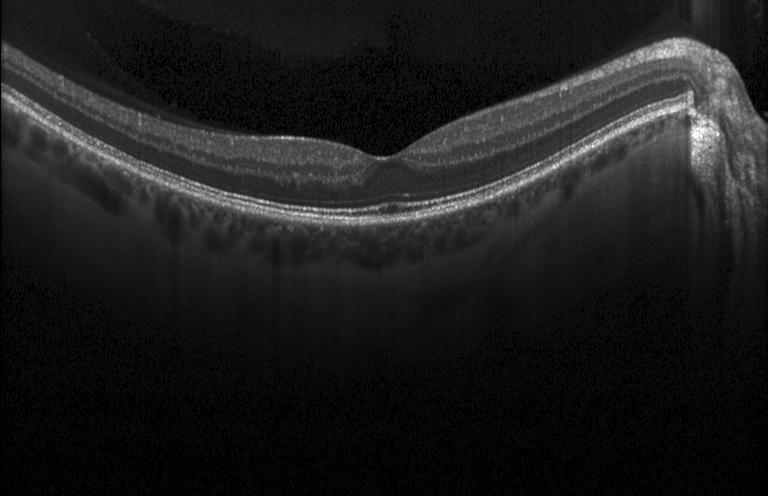
Heidelberg Spectralis OCT system · optical coherence tomography B-scan · fovea-centered · spectral-domain OCT. Finding: no evidence of CNV, DME, or drusen.